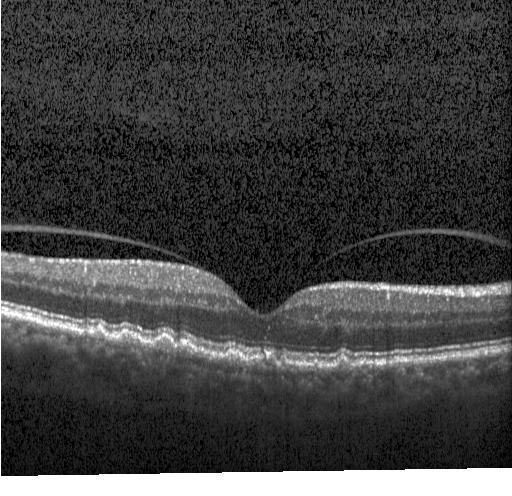 Spectral-domain optical coherence tomography. Heidelberg Spectralis. Horizontal scan through the fovea. OCT B-scan. Impression: multiple drusen.